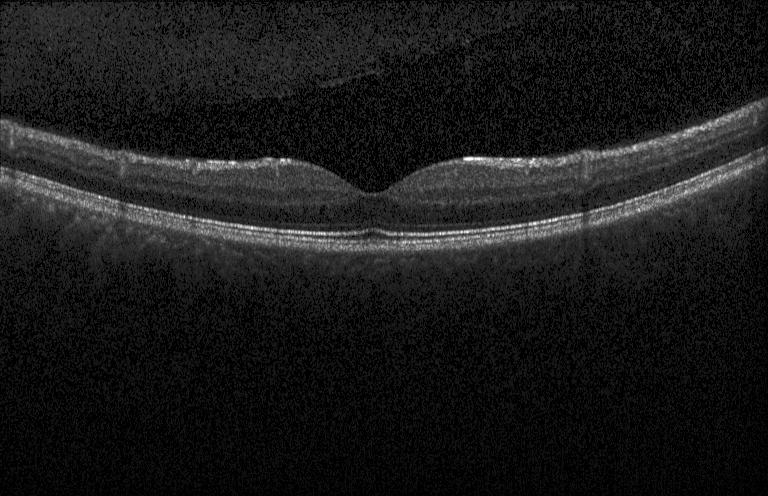 OCT finding: no evidence of CNV, DME, or drusen.